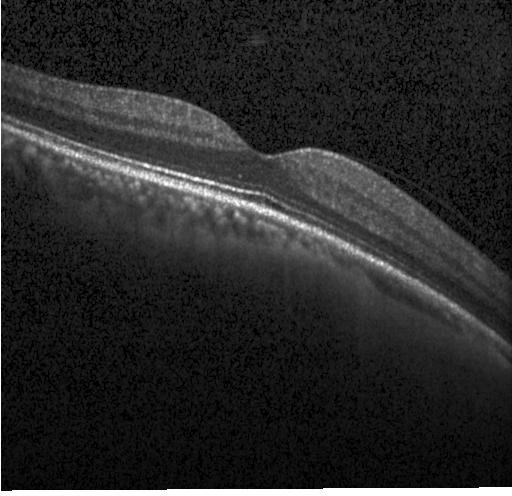

Instrument: Heidelberg Spectralis. Fovea-centered. Retinal OCT B-scan
The scan shows no choroidal neovascularization, no diabetic macular edema, and no drusen.